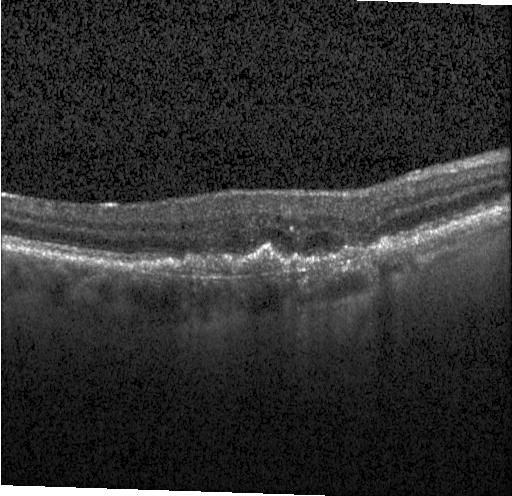

Macular scan. Instrument: Heidelberg Spectralis. Retinal OCT cross-section. Spectral-domain OCT
Finding: choroidal neovascularization.